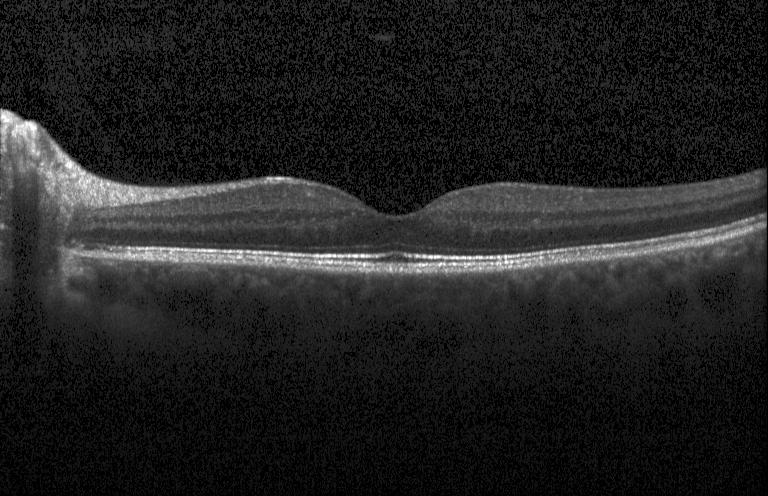 SD-OCT, fovea-centered, retinal OCT cross-section
The scan shows no CNV, no DME, and no drusen.